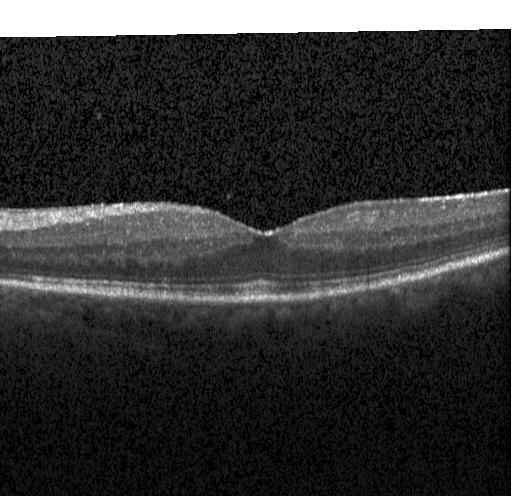
Impression: neither CNV, DME, nor drusen.